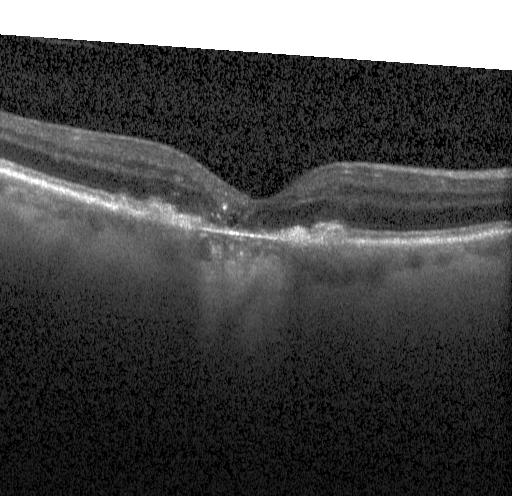

Retinal OCT cross-section
Diagnosis: CNV.